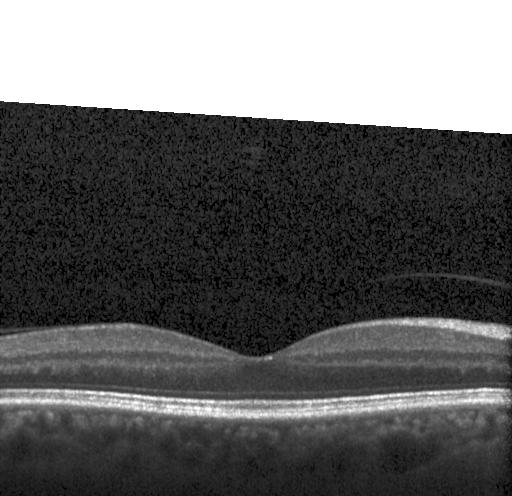
OCT B-scan, spectral-domain optical coherence tomography — OCT finding: neither CNV, DME, nor drusen.